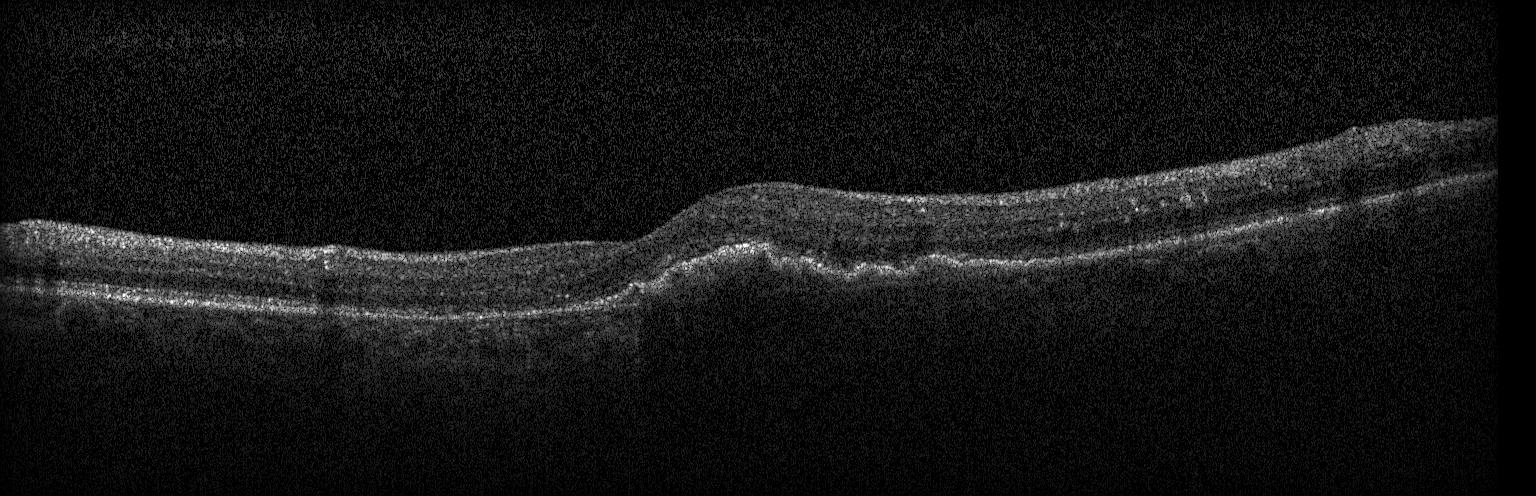
Macular scan, OCT line scan.
Diagnosis: a choroidal neovascular membrane.